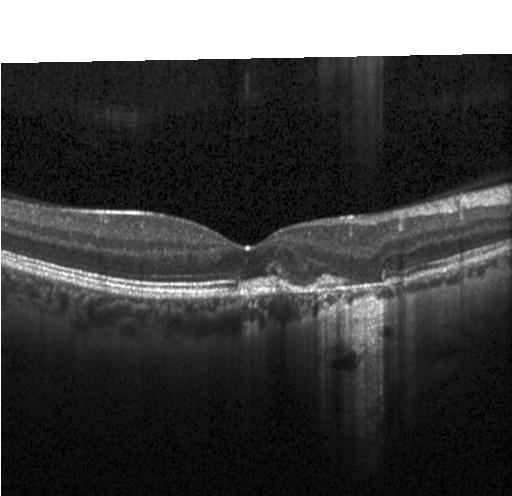
Impression: choroidal neovascularization.